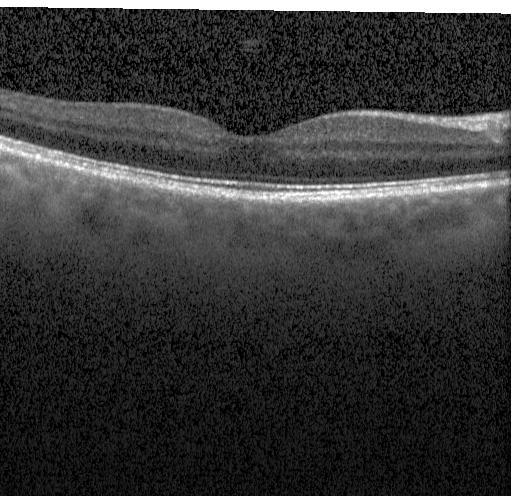

OCT line scan. Assessment: neither choroidal neovascularization, diabetic macular edema, nor drusen.